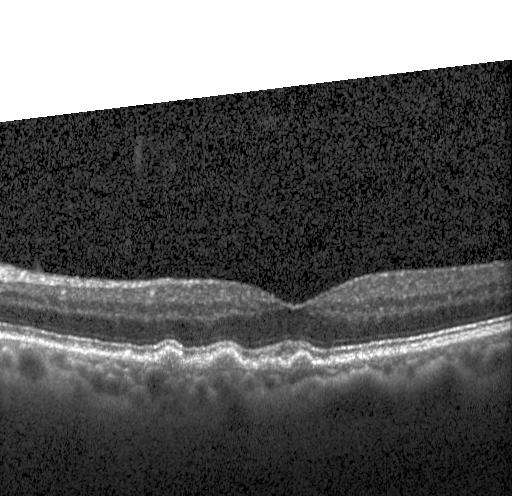
OCT line scan — Diagnosis: sub-RPE drusenoid deposits.